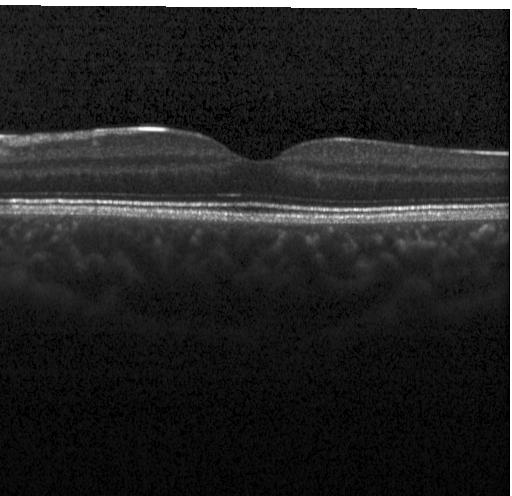 Diagnosis: no choroidal neovascularization, diabetic macular edema, or drusen.